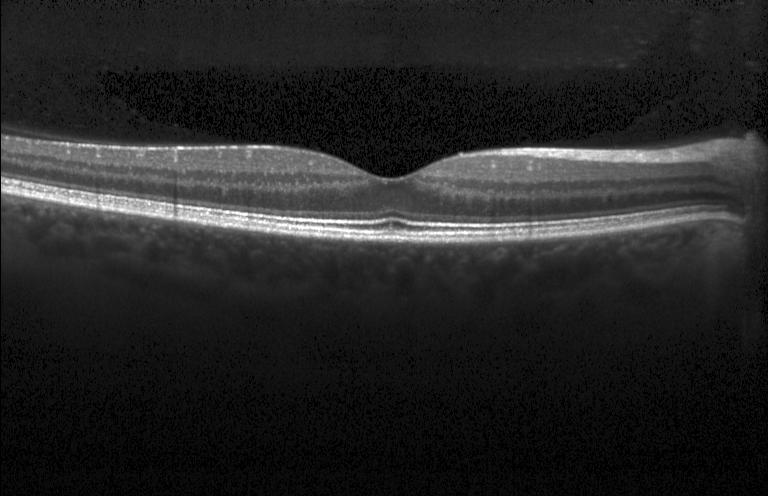 Instrument: Heidelberg Spectralis, spectral-domain optical coherence tomography, OCT line scan.
Impression: no choroidal neovascularization, diabetic macular edema, or drusen.